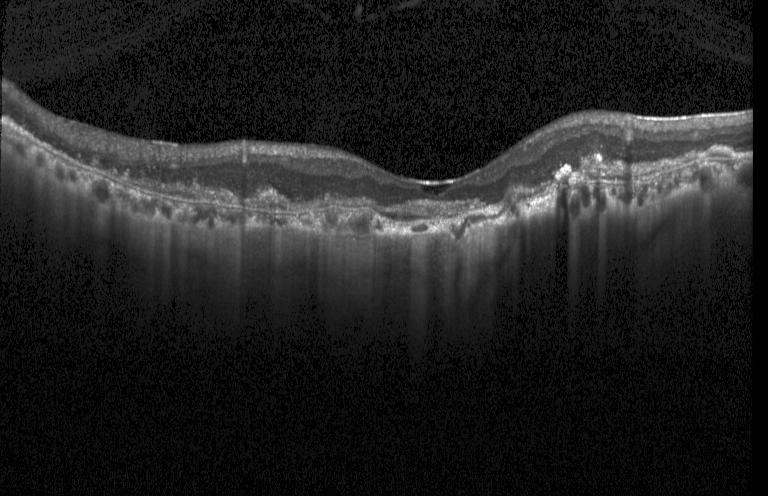 OCT B-scan showing a choroidal neovascular membrane.